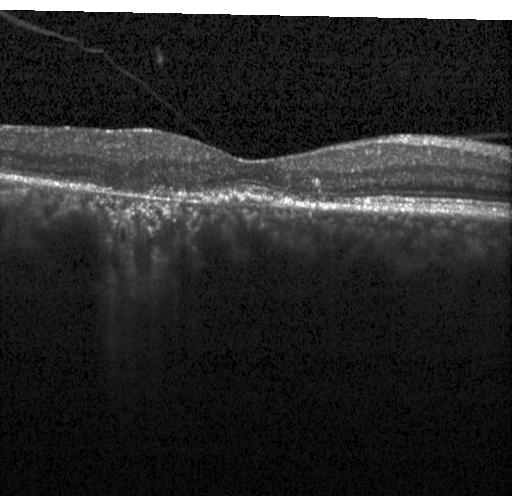

OCT finding: a choroidal neovascular membrane.